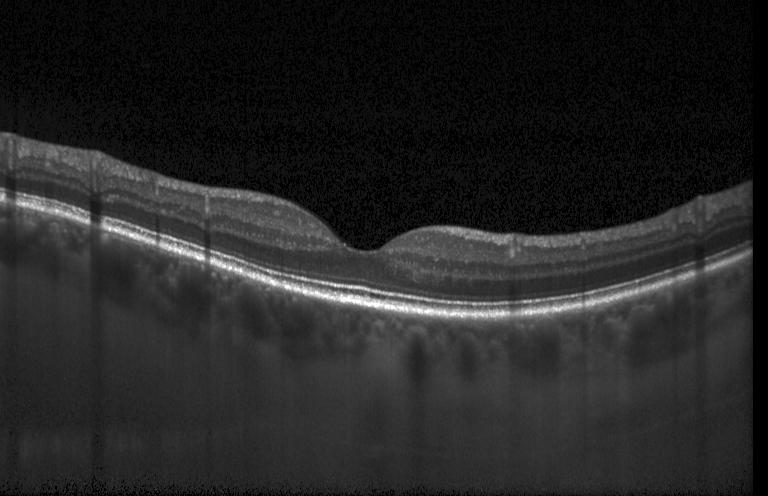
Finding: no CNV, DME, or drusen.